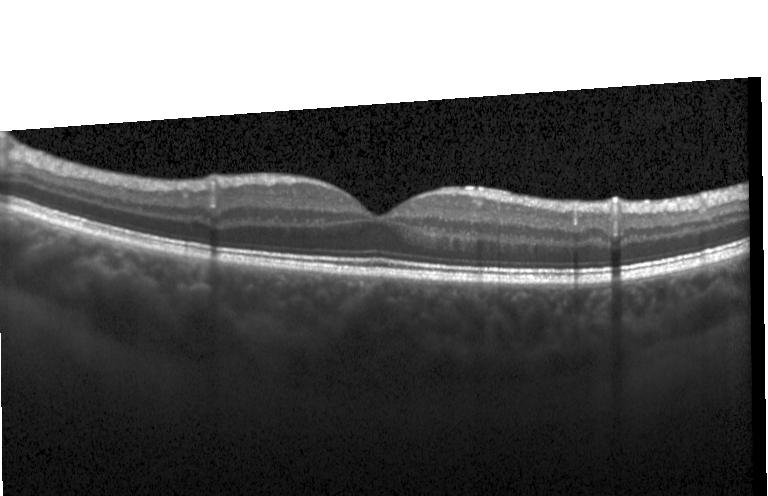

This B-scan demonstrates neither choroidal neovascularization, diabetic macular edema, nor drusen.